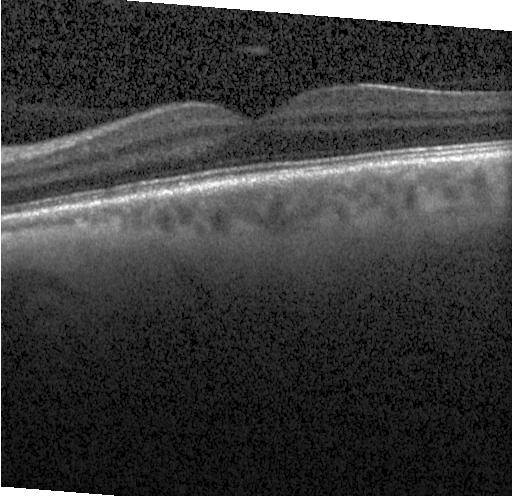
OCT scan showing no CNV, no DME, and no drusen.